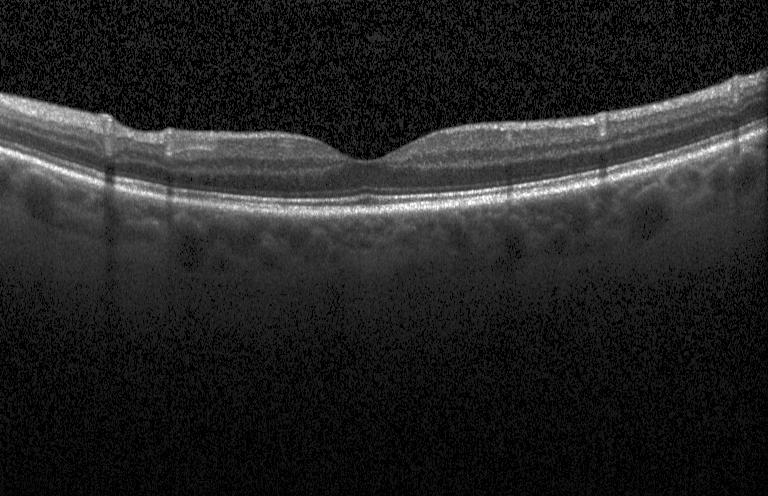 Finding: no CNV, DME, or drusen.